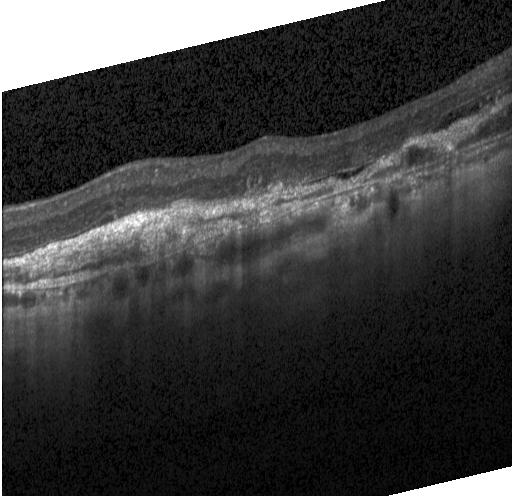

OCT finding: a choroidal neovascular membrane.